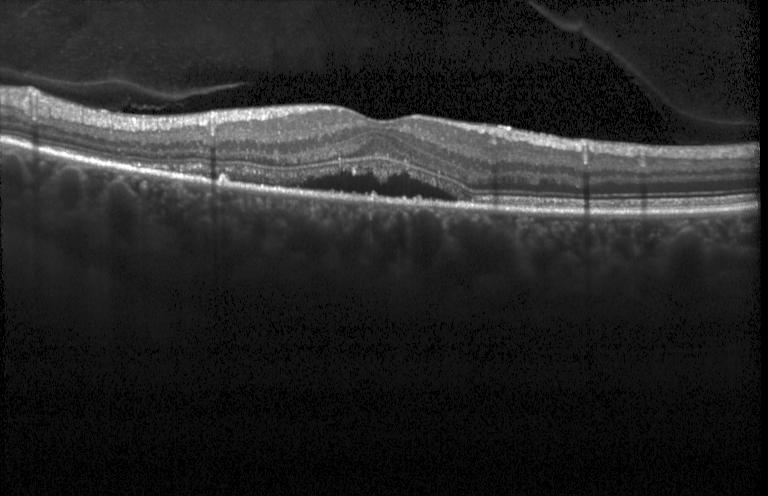 OCT B-scan; spectral-domain OCT; instrument: Heidelberg Spectralis. CNV.